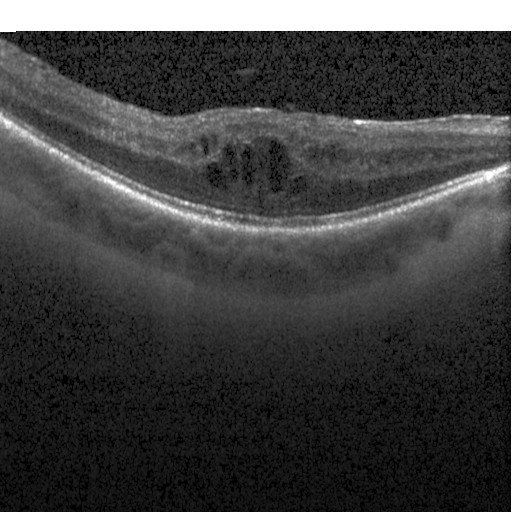
Impression: diabetic macular edema.